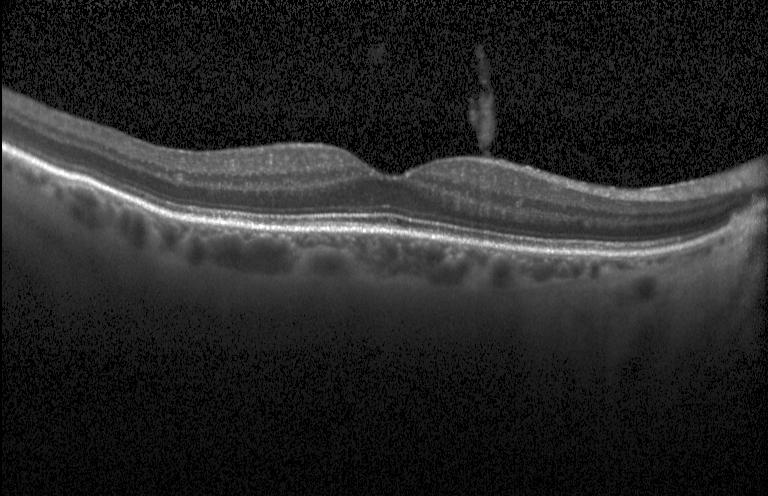
OCT B-scan; spectral-domain OCT
Finding: no choroidal neovascularization, no diabetic macular edema, and no drusen.